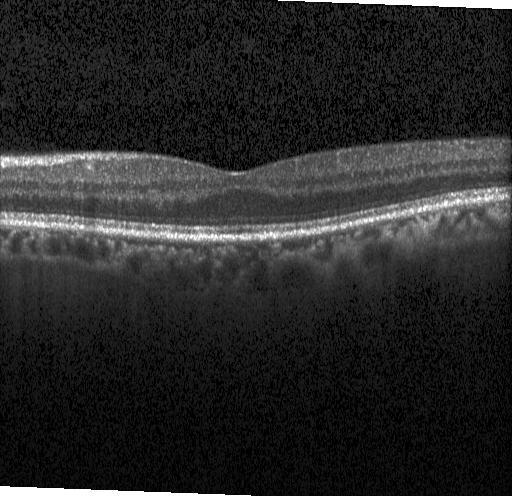

Through the macula. OCT line scan.
Impression: no evidence of CNV, DME, or drusen.